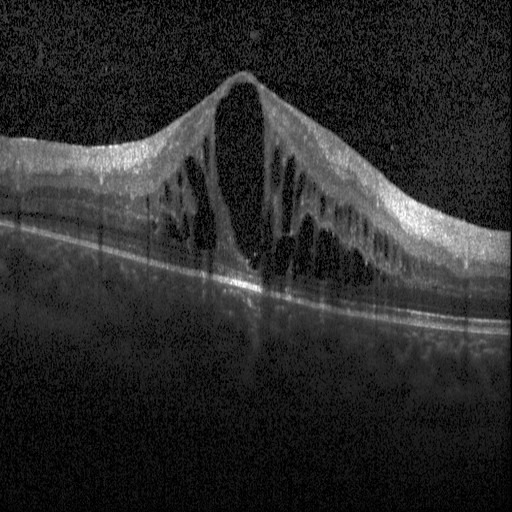 SD-OCT · retinal OCT cross-section · through the macula.
Impression: diabetic macular edema (DME).